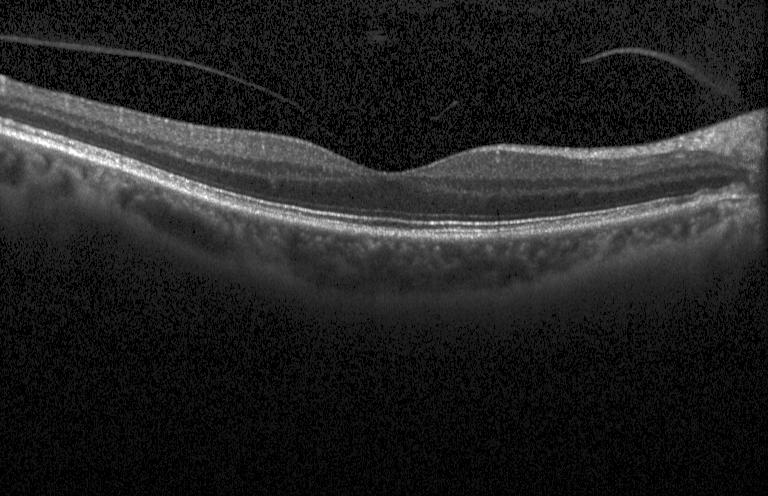 Fovea-centered; retinal OCT cross-section
Finding: neither choroidal neovascularization, diabetic macular edema, nor drusen.